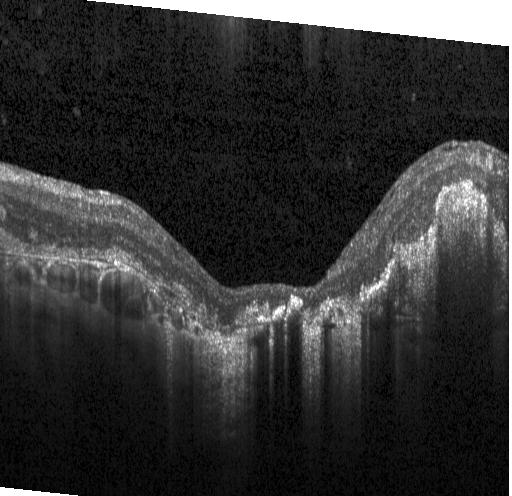
Impression: choroidal neovascularization.